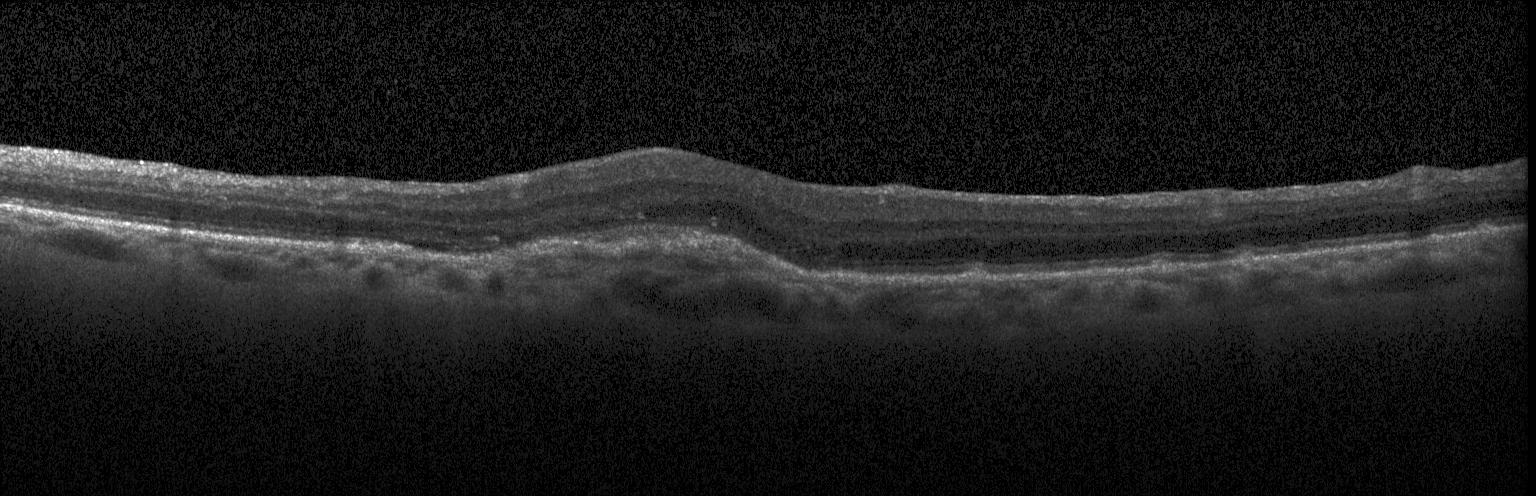
Acquired on a Heidelberg Spectralis, optical coherence tomography scan.
Diagnosis: CNV.